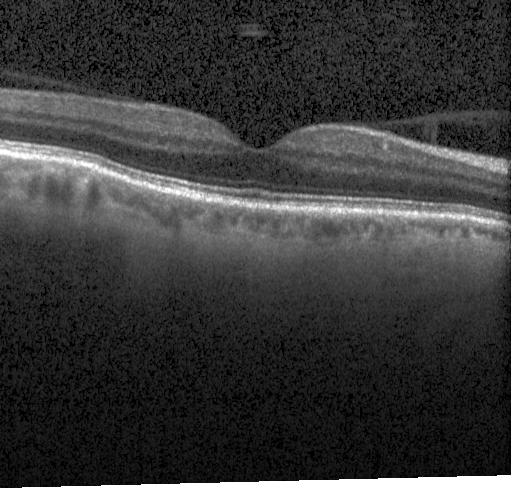 Retinal OCT B-scan · Heidelberg Spectralis OCT system. Dx: no CNV, DME, or drusen.